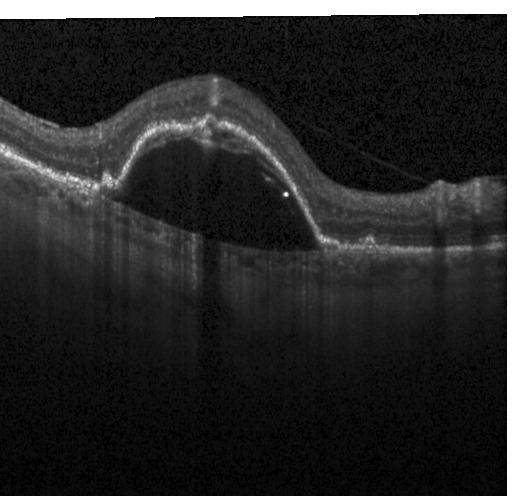

The scan shows choroidal neovascularization (CNV).